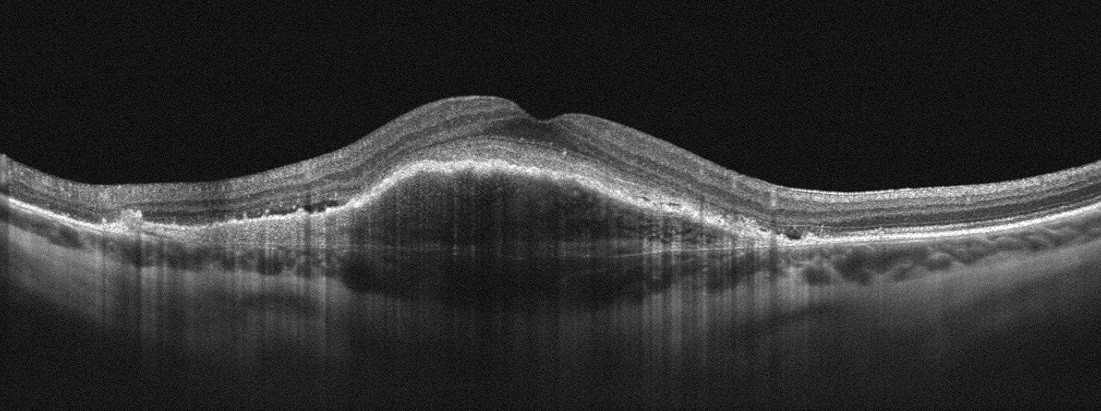 Impression: age-related macular degeneration.